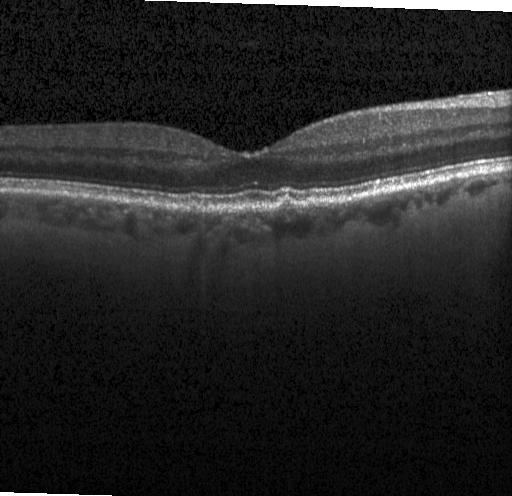
OCT B-scan — Macular OCT: drusen.